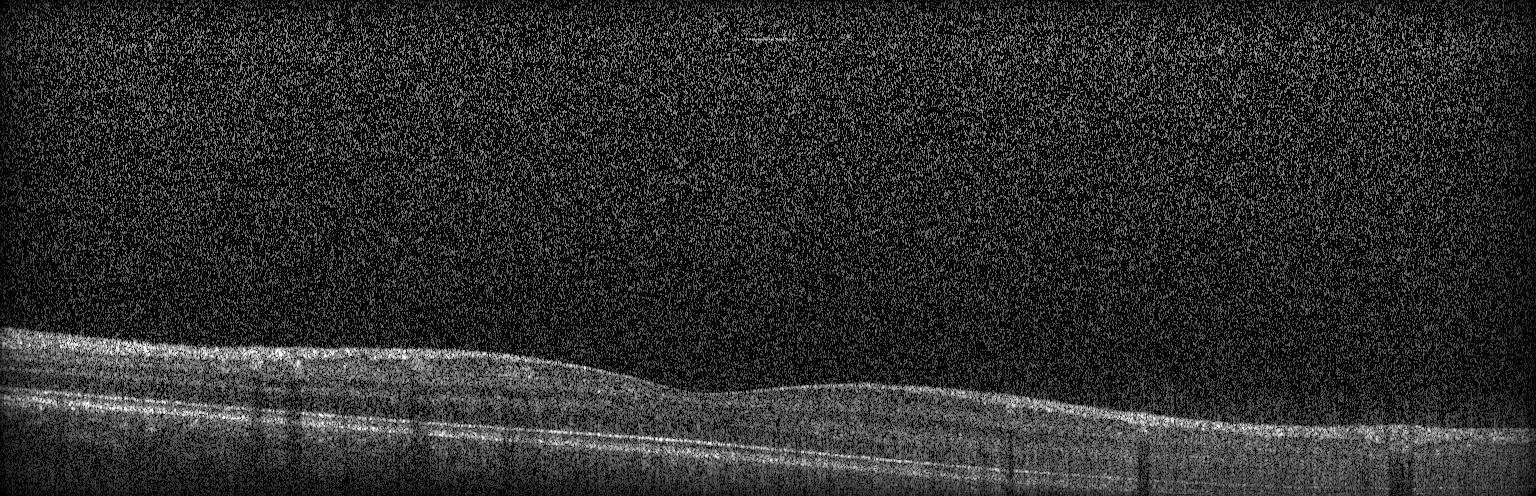

Spectral-domain OCT B-scan: no choroidal neovascularization, no diabetic macular edema, and no drusen.